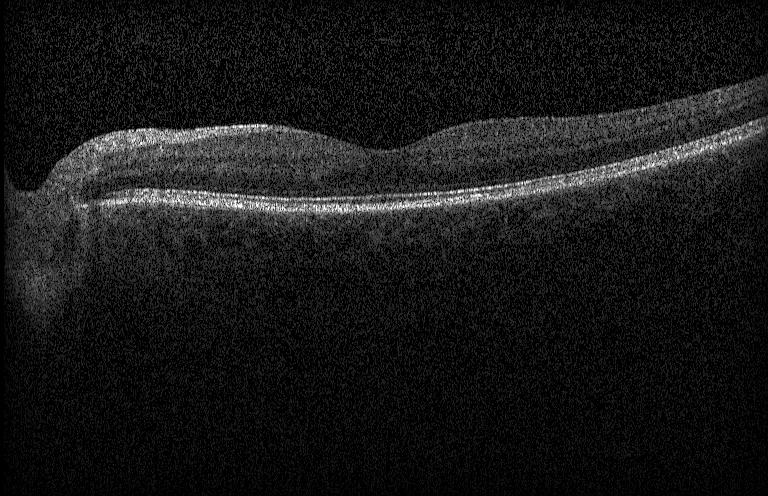

Impression: no evidence of choroidal neovascularization, diabetic macular edema, or drusen.